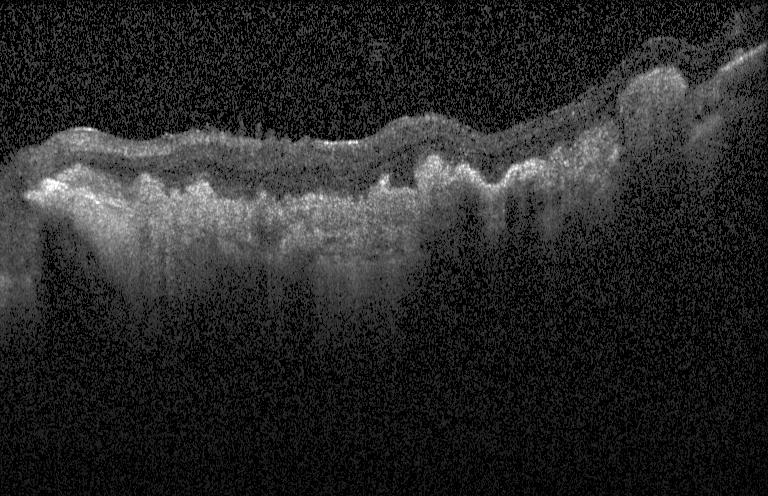 Assessment: a choroidal neovascular membrane.